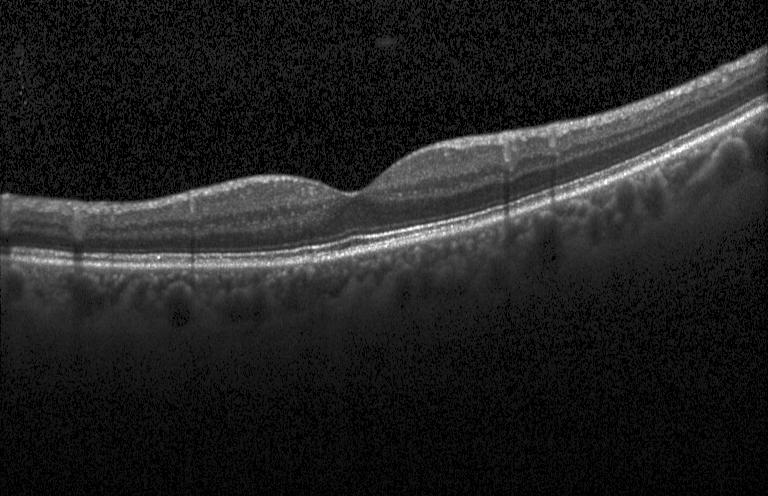 Retinal OCT B-scan, through the macula, spectral-domain OCT, acquired on a Heidelberg Spectralis — Impression: no evidence of CNV, DME, or drusen.